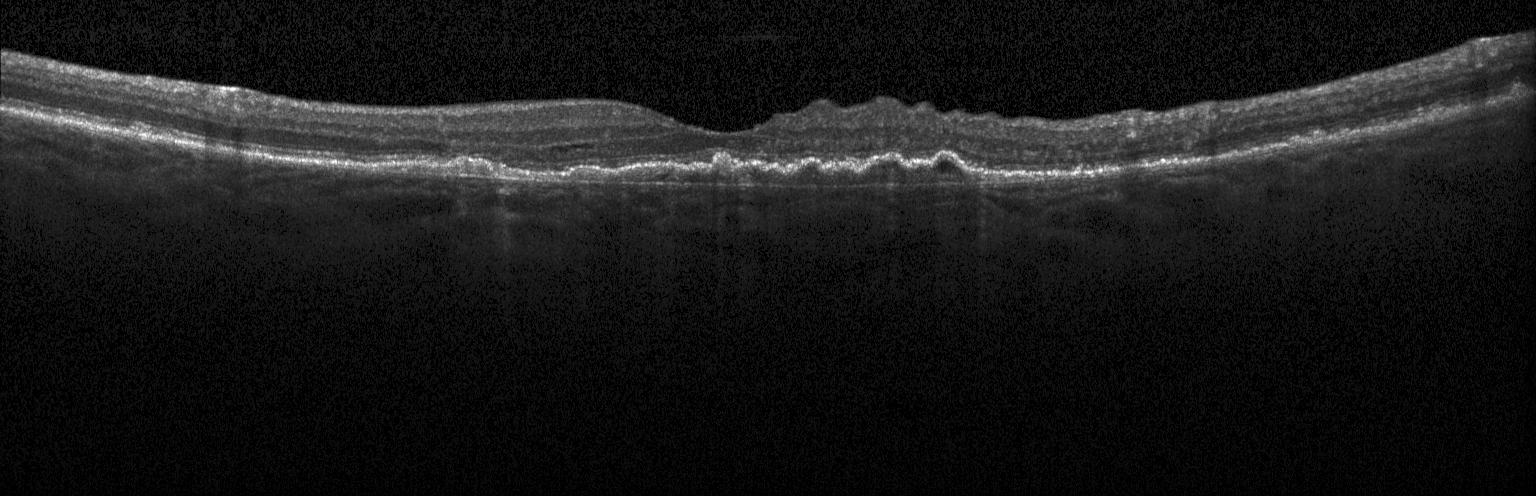 The scan shows choroidal neovascularization.